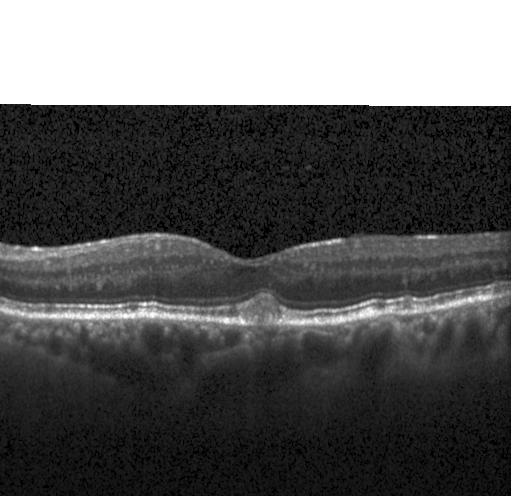

SD-OCT · acquired on a Heidelberg Spectralis · retinal OCT B-scan.
Finding: multiple drusen.